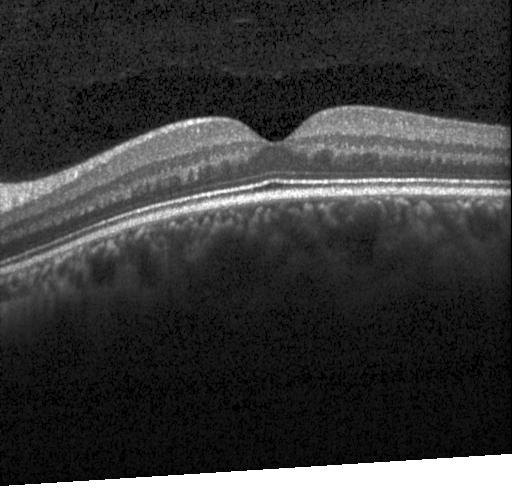 Macular OCT demonstrating no evidence of choroidal neovascularization, diabetic macular edema, or drusen.